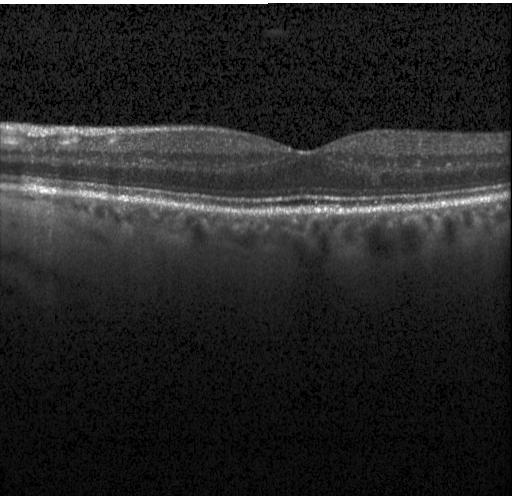
OCT line scan · SD-OCT · instrument: Heidelberg Spectralis · horizontal scan through the fovea — Finding: no evidence of choroidal neovascularization, diabetic macular edema, or drusen.